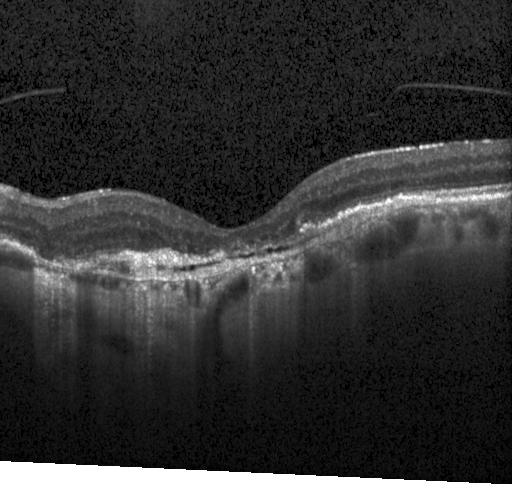
Heidelberg Spectralis · optical coherence tomography B-scan · SD-OCT.
A choroidal neovascular membrane.